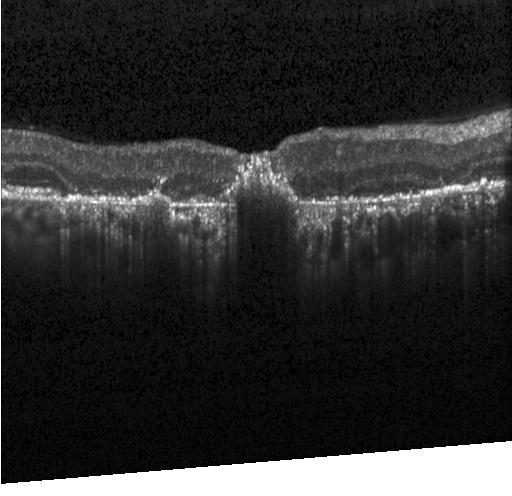 Macular scan · optical coherence tomography B-scan. Finding: a choroidal neovascular membrane.